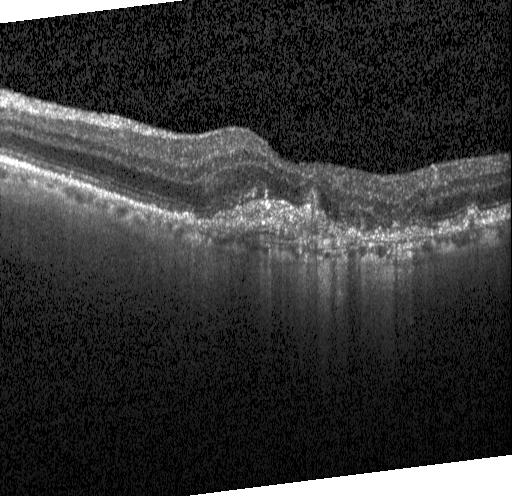

Spectral-domain OCT, through the macula, retinal OCT cross-section, Heidelberg Spectralis.
Assessment: choroidal neovascularization.